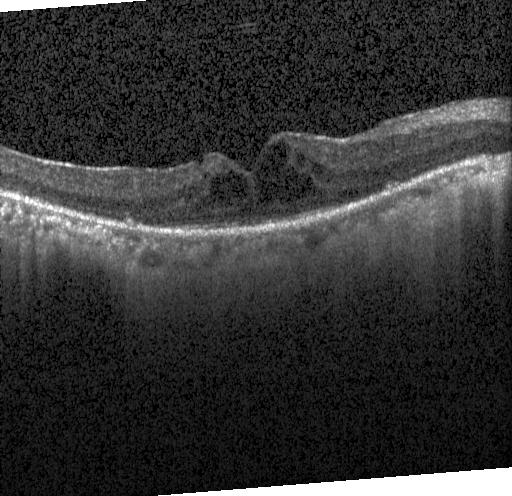
Retinal OCT B-scan. Centered on the fovea — Impression: diabetic macular edema (DME).